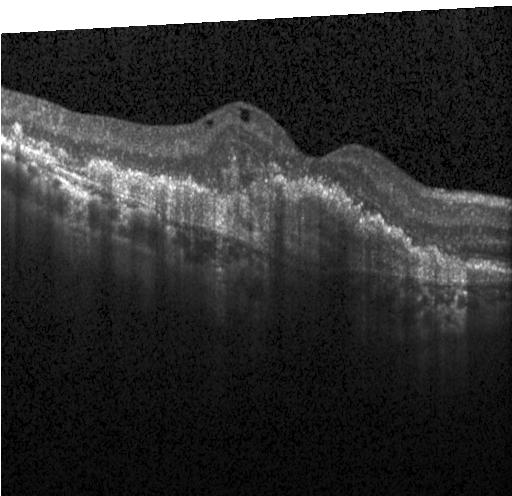
The scan shows choroidal neovascularization (CNV).